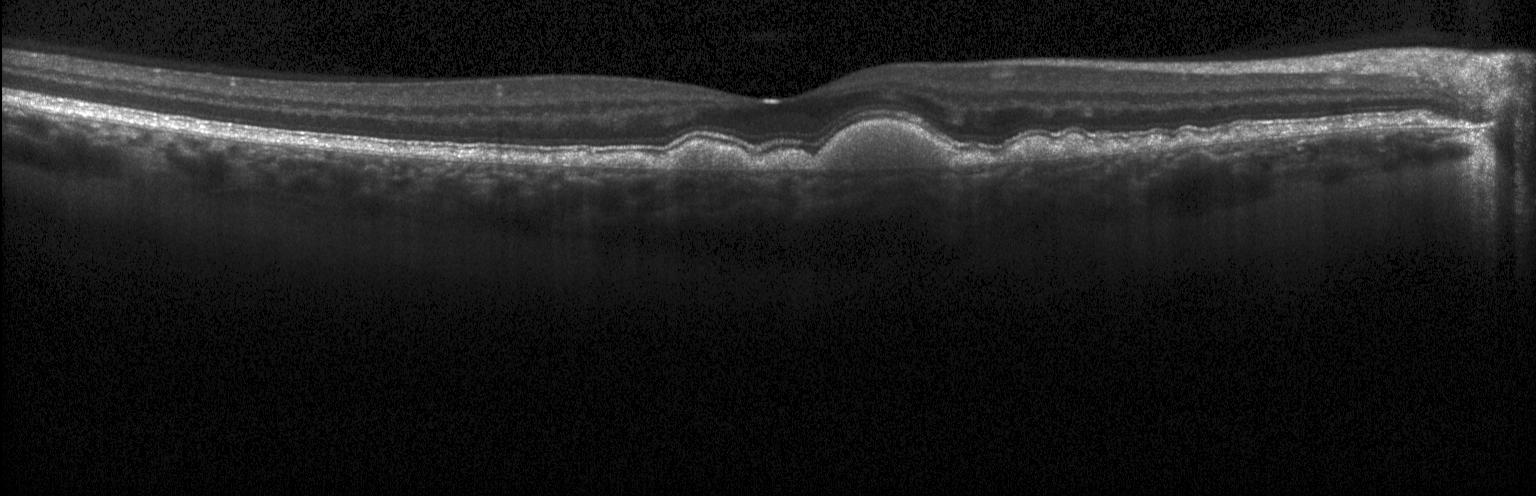 Retinal OCT B-scan, through the macula, SD-OCT, Heidelberg Spectralis OCT system.
The scan shows drusen.